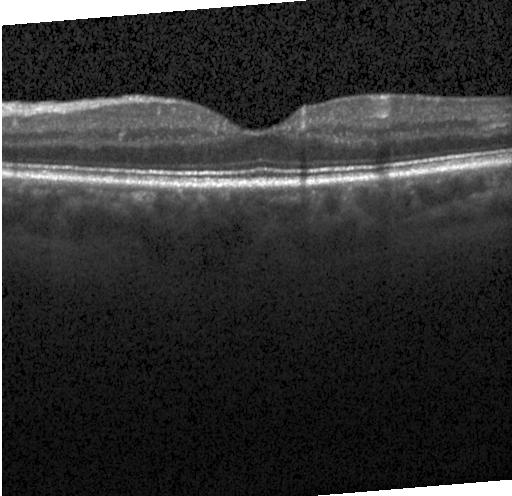 Diagnosis: neither CNV, DME, nor drusen.